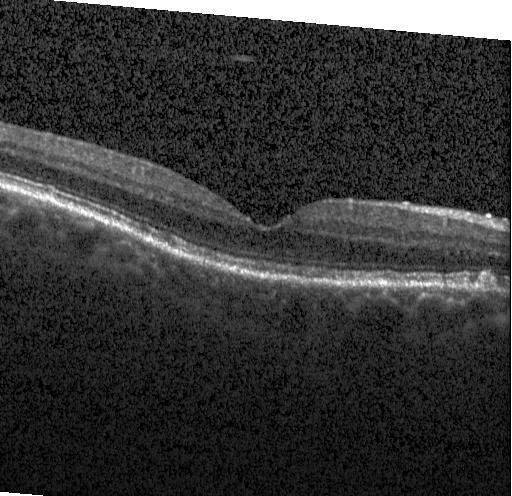
Optical coherence tomography scan. Spectral-domain OCT — Dx: drusen.